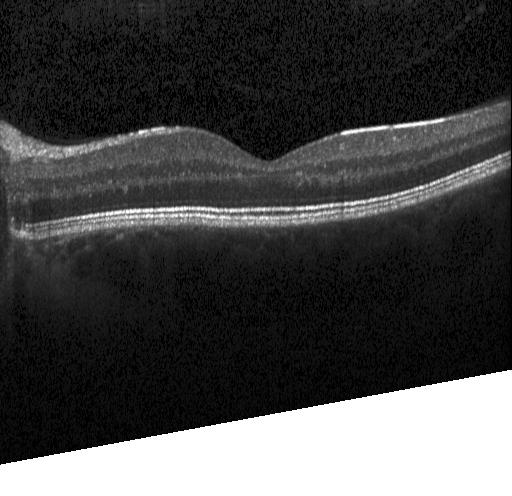
SD-OCT, retinal OCT cross-section, centered on the fovea, instrument: Heidelberg Spectralis.
OCT finding: no evidence of CNV, DME, or drusen.